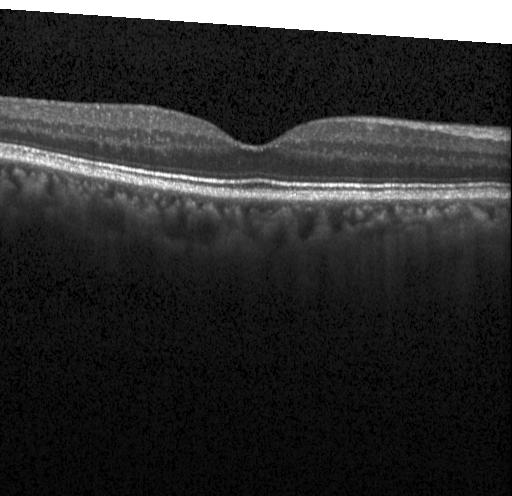
Finding: no choroidal neovascularization, diabetic macular edema, or drusen.